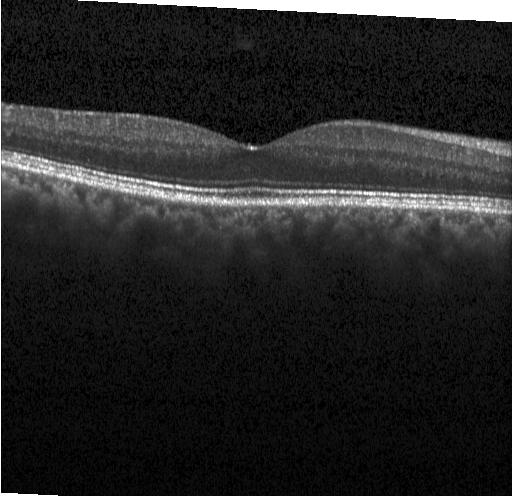
Optical coherence tomography B-scan.
Diagnosis: neither CNV, DME, nor drusen.